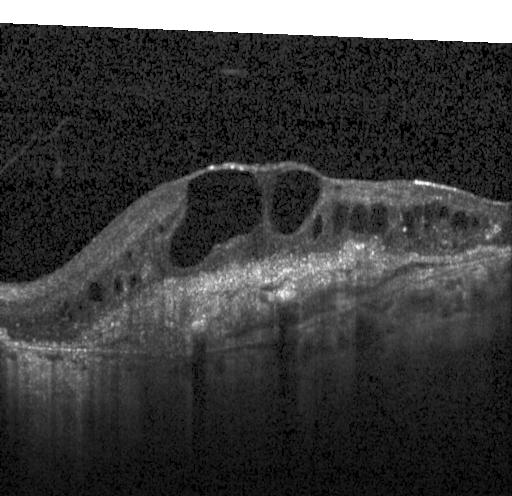 This B-scan demonstrates choroidal neovascularization.